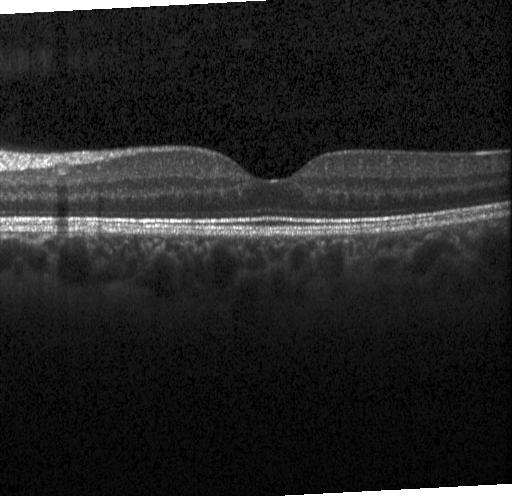

Spectral-domain optical coherence tomography, Heidelberg Spectralis, retinal OCT B-scan. Finding: no CNV, no DME, and no drusen.